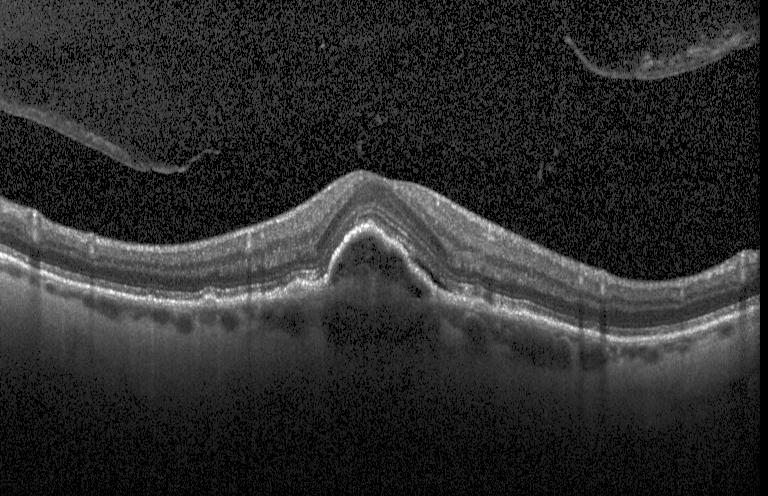

OCT B-scan.
Impression: choroidal neovascularization (CNV).